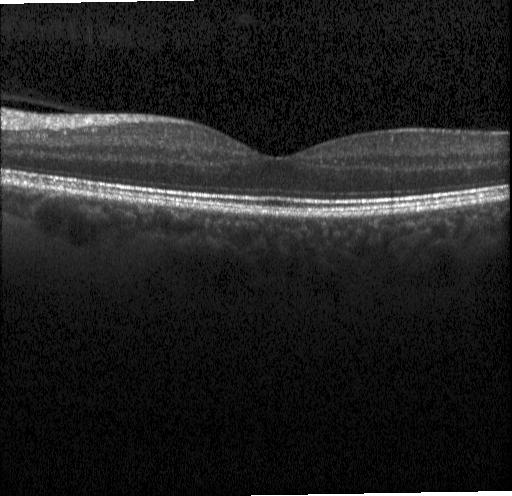 OCT line scan — Impression: no CNV, DME, or drusen.